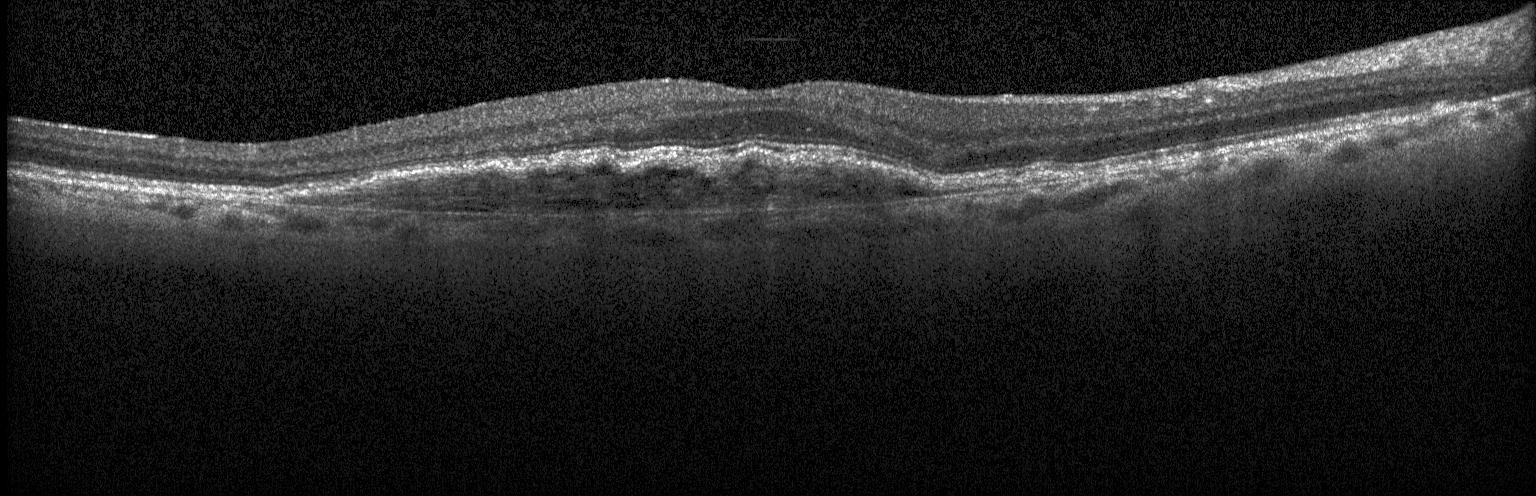 This B-scan demonstrates choroidal neovascularization.